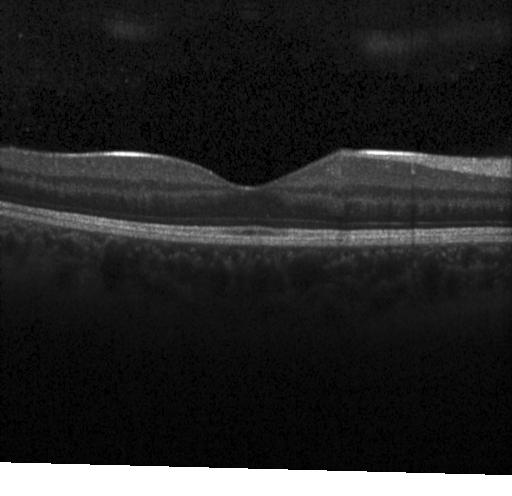 Finding: no choroidal neovascularization, diabetic macular edema, or drusen.